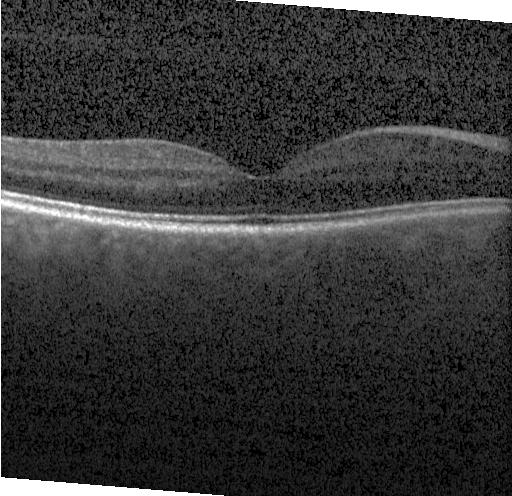
Assessment: neither CNV, DME, nor drusen.